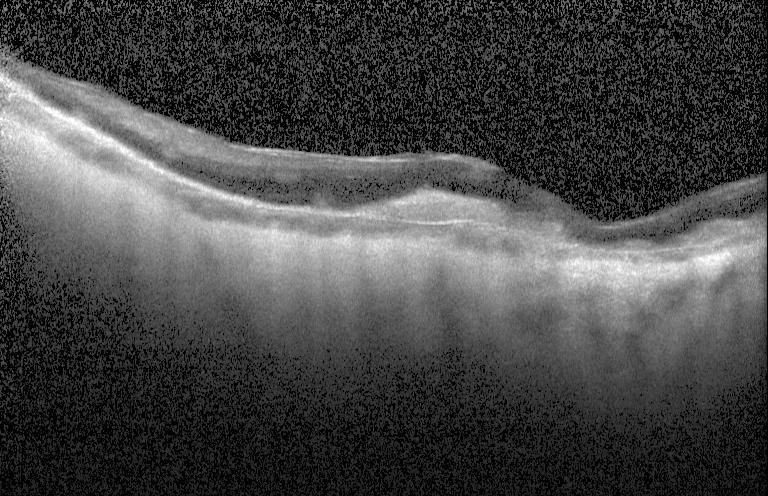 OCT line scan, Heidelberg Spectralis OCT system — Dx: choroidal neovascularization.